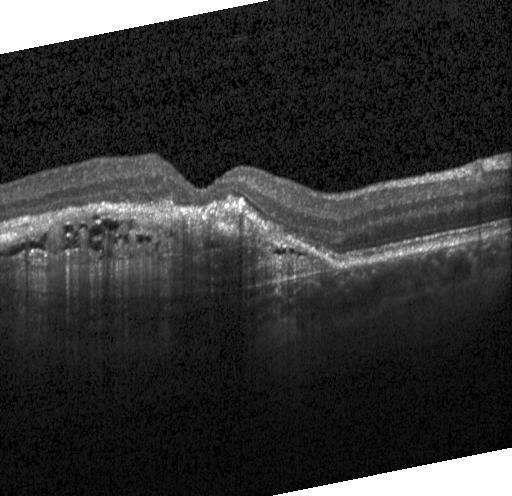

Optical coherence tomography scan; fovea-centered
Finding: a choroidal neovascular membrane.